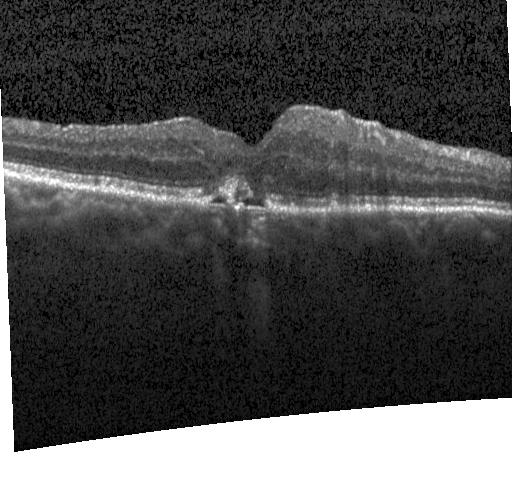
Retinal OCT B-scan
A choroidal neovascular membrane.